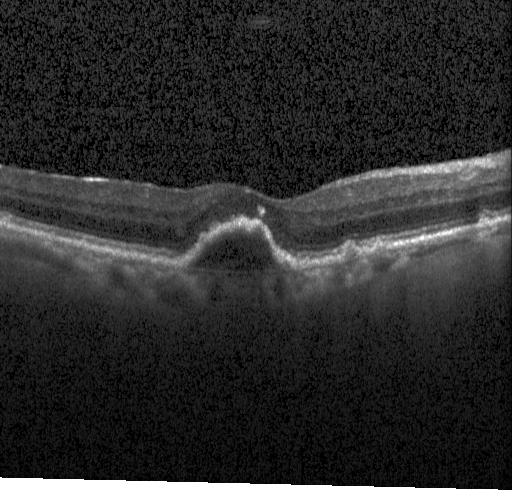

OCT finding: choroidal neovascularization (CNV).